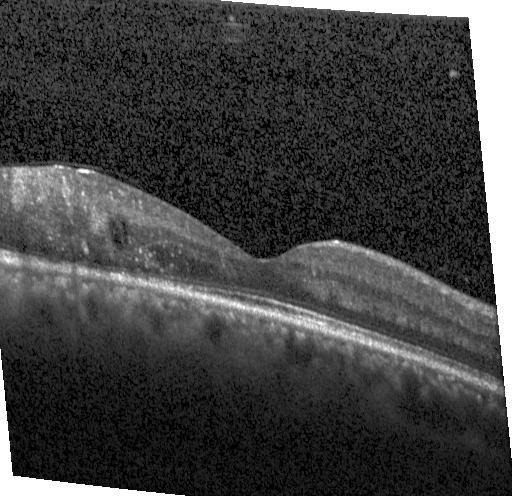 OCT finding: diabetic macular edema.